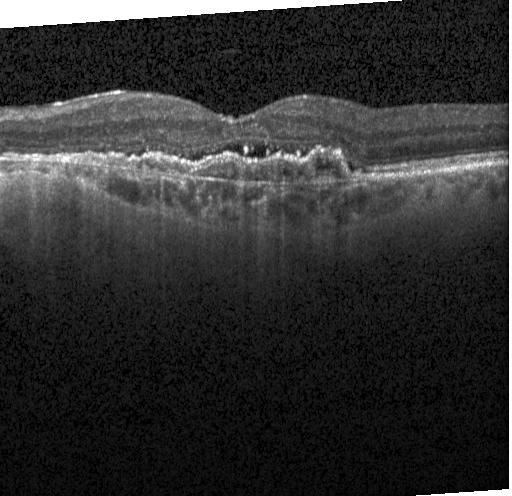 Heidelberg Spectralis OCT system, OCT B-scan, spectral-domain optical coherence tomography, macular scan. Impression: CNV.